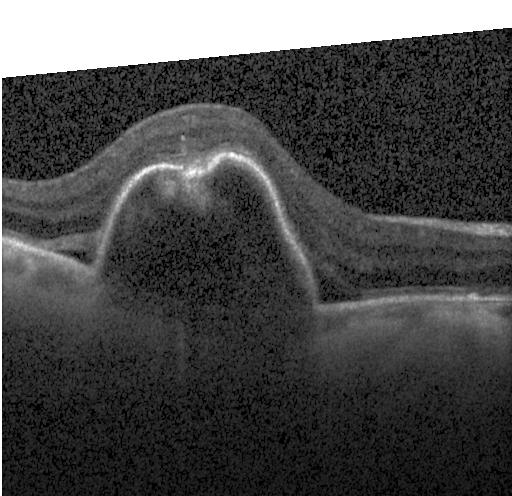
Heidelberg Spectralis OCT system · OCT line scan — Assessment: a choroidal neovascular membrane.